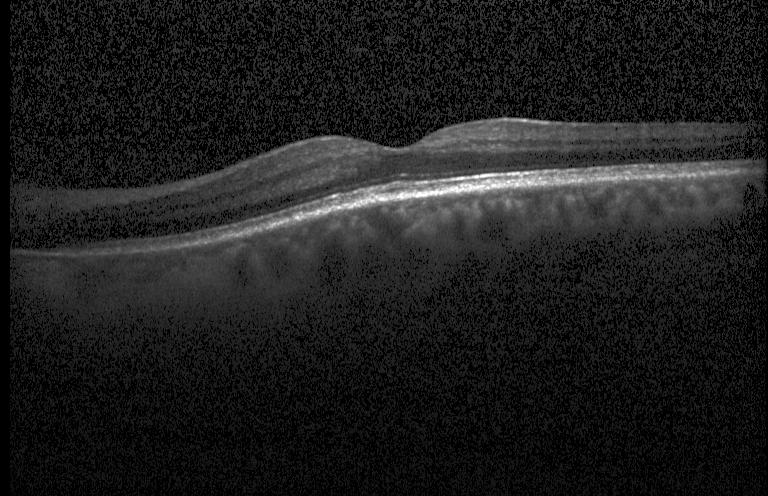
Impression: neither choroidal neovascularization, diabetic macular edema, nor drusen.